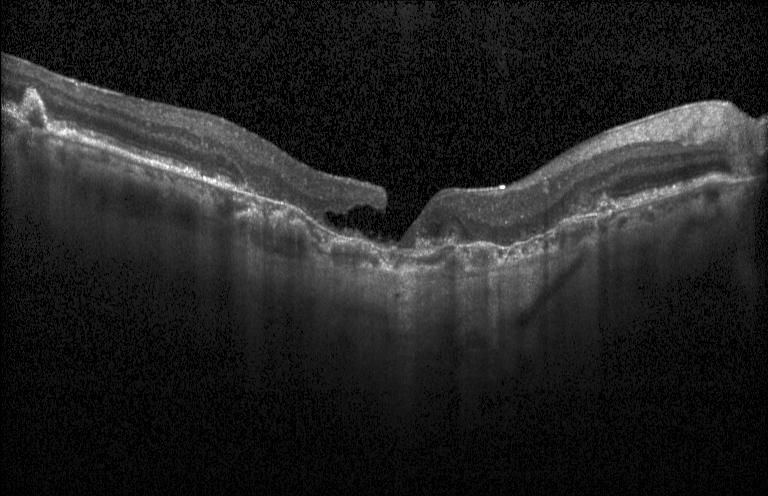
Finding: a choroidal neovascular membrane.